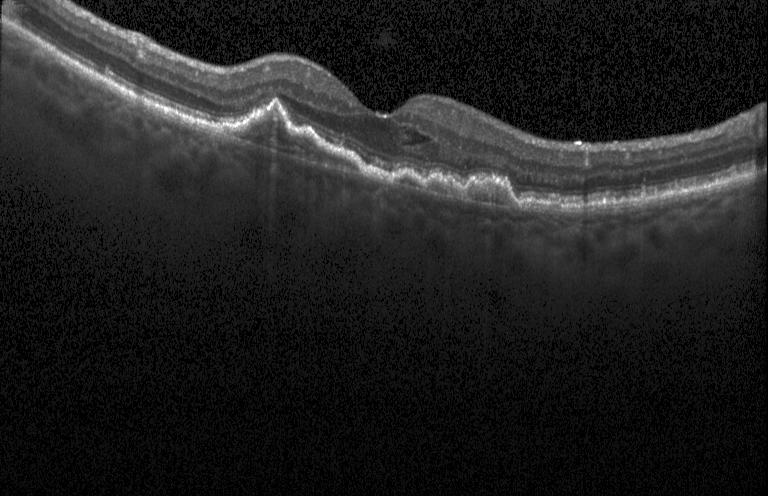

Macular scan, spectral-domain optical coherence tomography, OCT line scan, instrument: Heidelberg Spectralis.
This B-scan demonstrates a choroidal neovascular membrane.